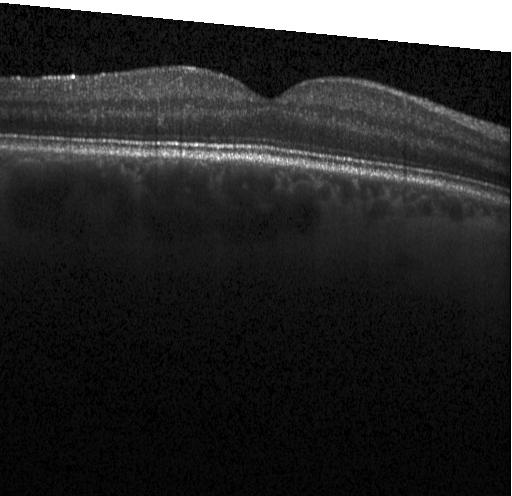
Heidelberg Spectralis · retinal OCT cross-section. Dx: no choroidal neovascularization, no diabetic macular edema, and no drusen.